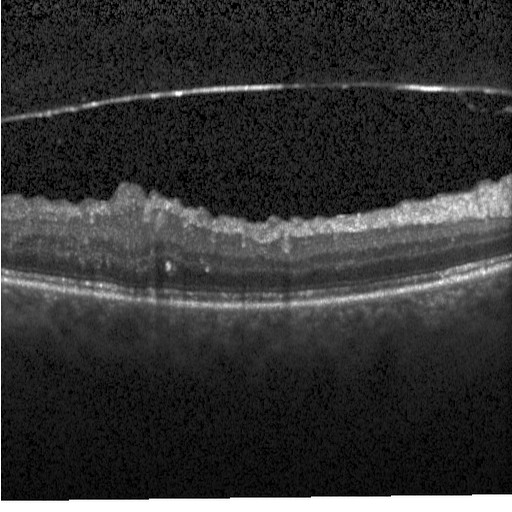

Finding: diabetic macular edema.